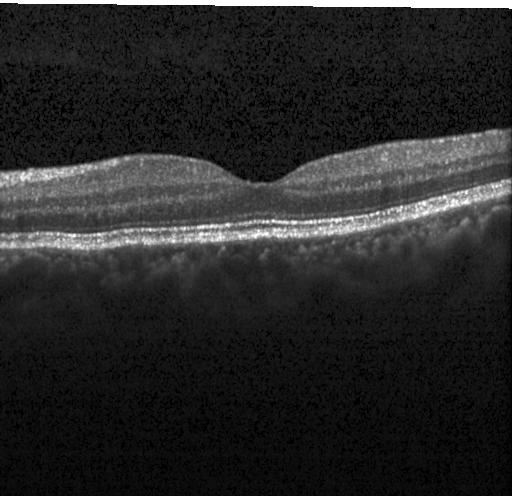

OCT line scan
Finding: no CNV, no DME, and no drusen.